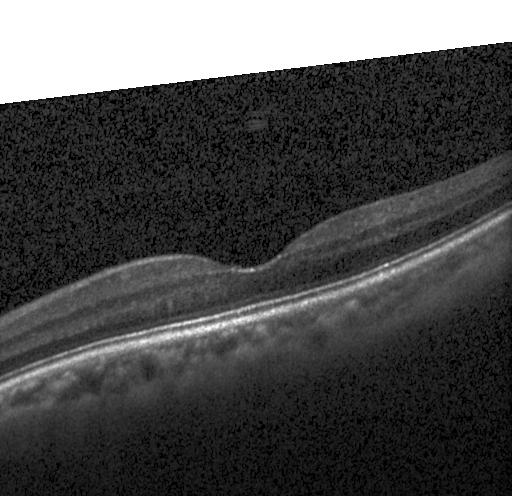
OCT B-scan.
No choroidal neovascularization, no diabetic macular edema, and no drusen.